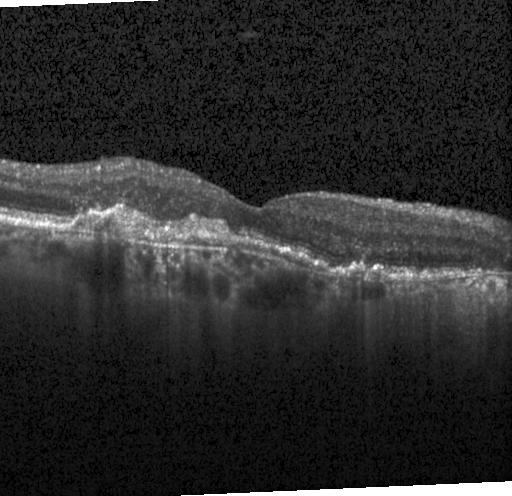 Diagnosis: a choroidal neovascular membrane.